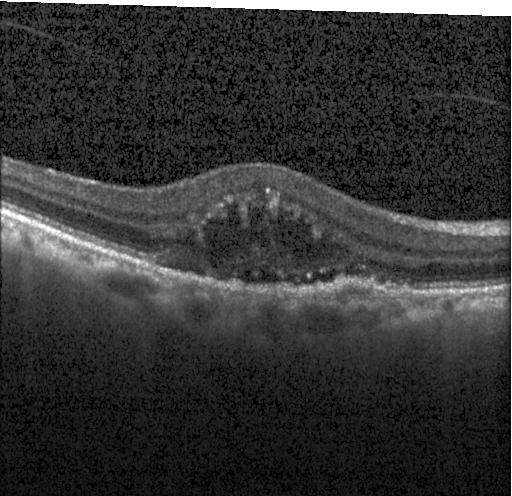
Heidelberg Spectralis OCT system; optical coherence tomography B-scan. Macular OCT: choroidal neovascularization.